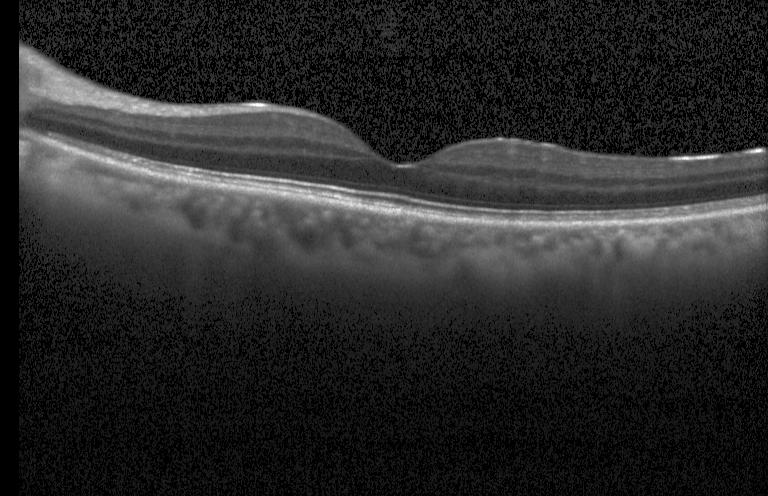 OCT B-scan · spectral-domain optical coherence tomography · fovea-centered — Finding: neither choroidal neovascularization, diabetic macular edema, nor drusen.